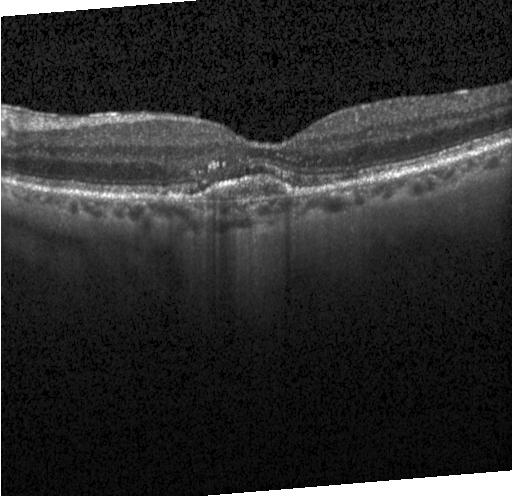 Retinal OCT cross-section. SD-OCT. Macular scan
Finding: a choroidal neovascular membrane.